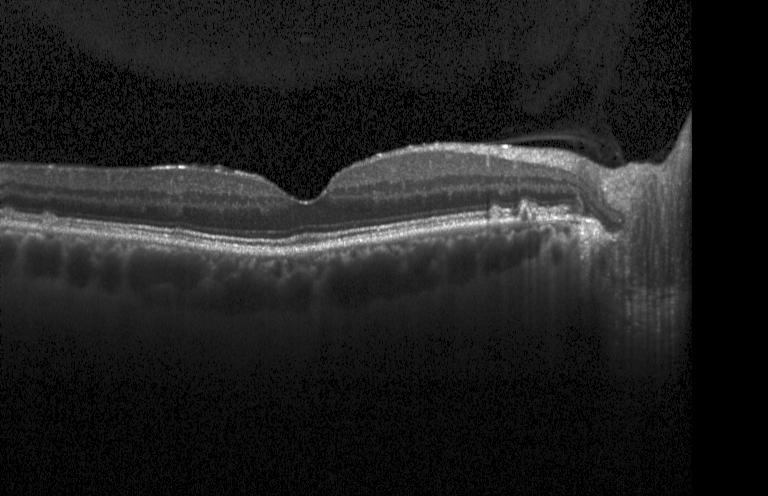

OCT line scan.
This B-scan demonstrates drusen.